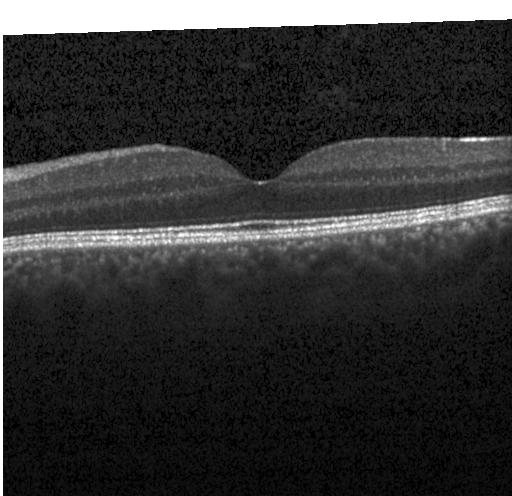 No choroidal neovascularization, no diabetic macular edema, and no drusen.